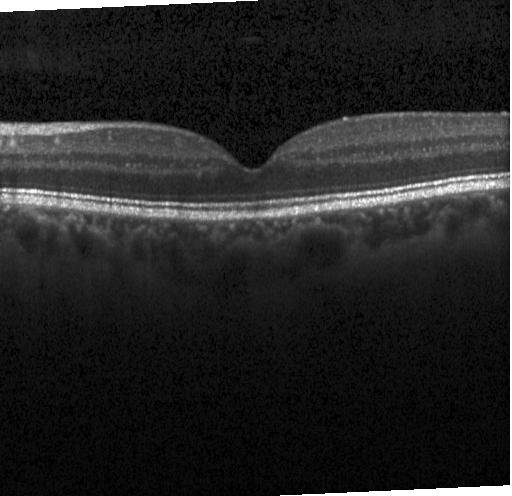

No choroidal neovascularization, diabetic macular edema, or drusen.